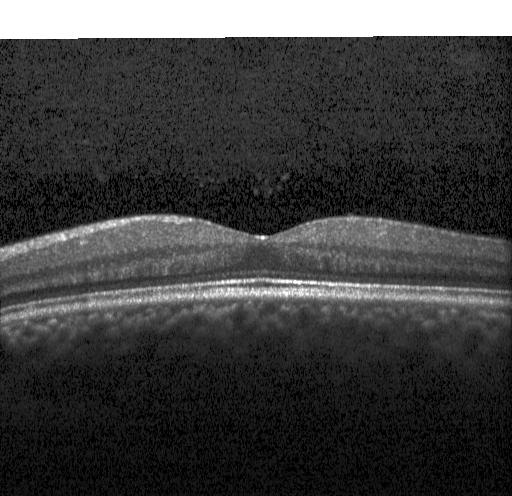
Assessment: no choroidal neovascularization, no diabetic macular edema, and no drusen.